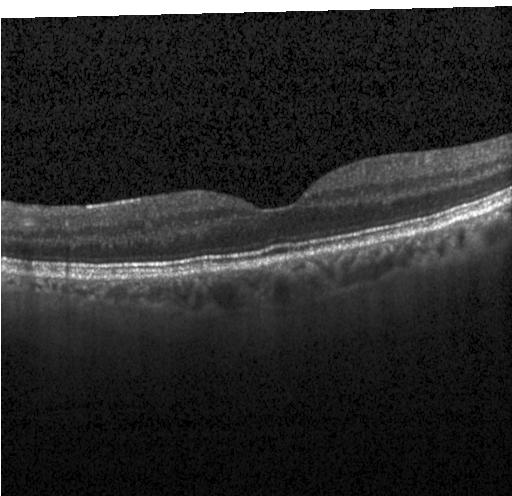 Spectral-domain OCT B-scan: no choroidal neovascularization, no diabetic macular edema, and no drusen.